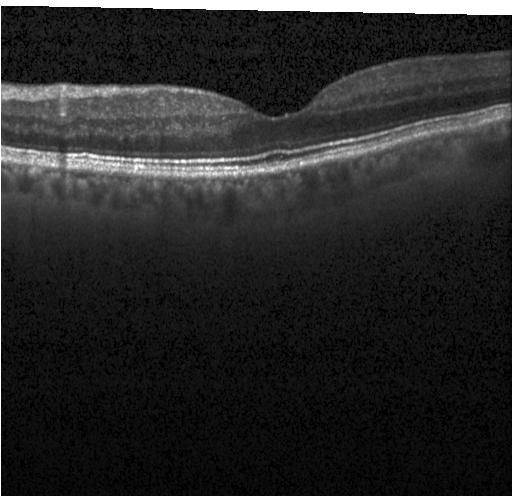 Retinal OCT B-scan; spectral-domain OCT
OCT finding: neither CNV, DME, nor drusen.